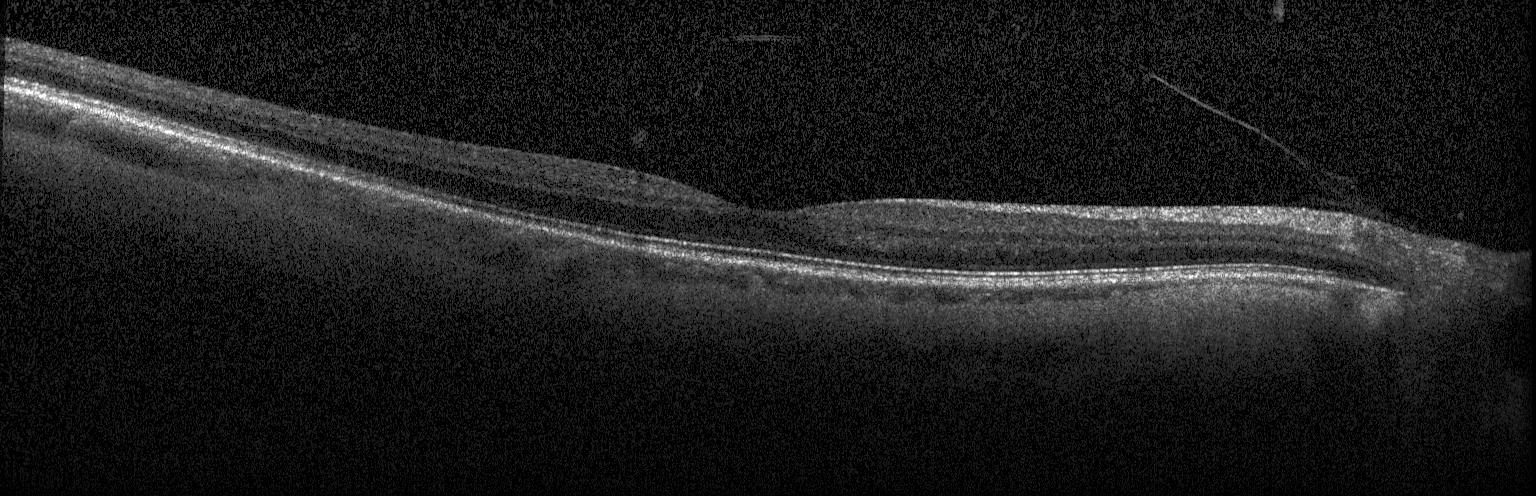
OCT B-scan · spectral-domain OCT
This B-scan demonstrates neither CNV, DME, nor drusen.